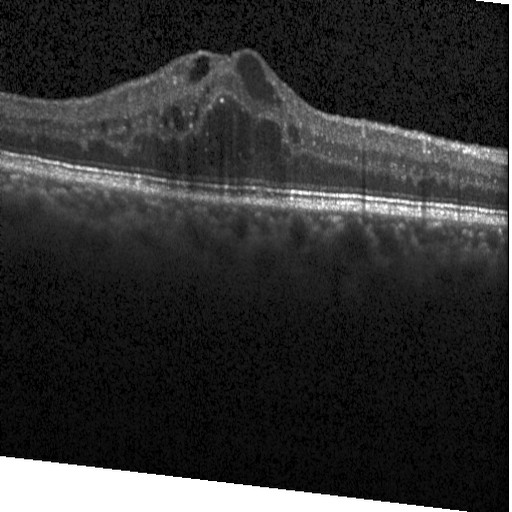

Optical coherence tomography scan; spectral-domain OCT; macular scan.
Diabetic macular edema.